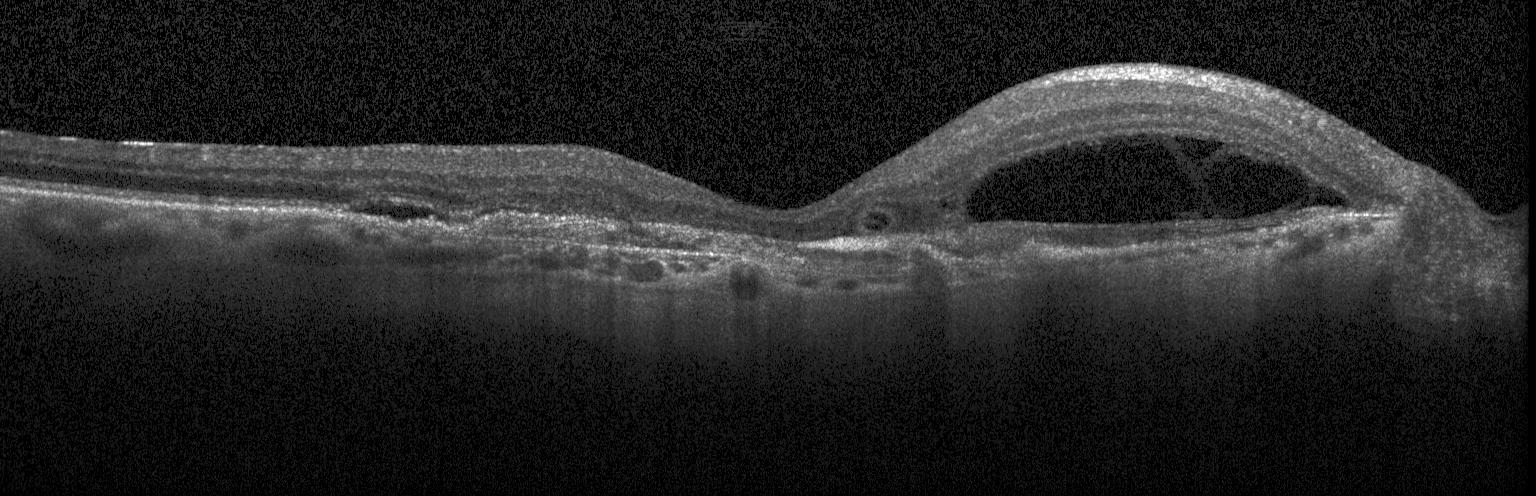 Optical coherence tomography B-scan — Impression: choroidal neovascularization (CNV).